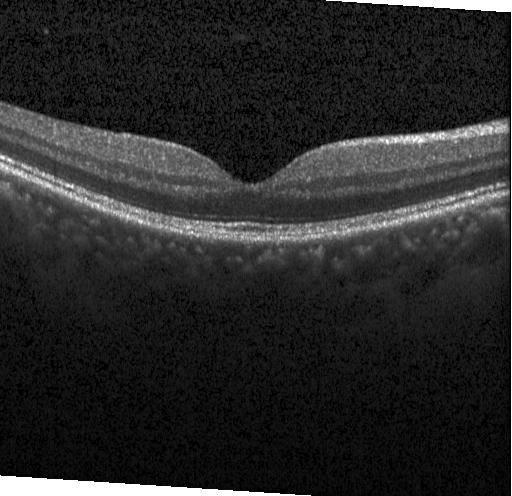
Optical coherence tomography scan — Finding: no CNV, no DME, and no drusen.